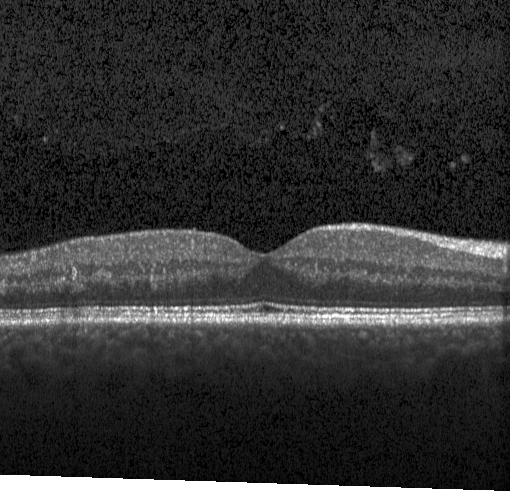 Heidelberg Spectralis OCT system; OCT line scan; spectral-domain optical coherence tomography; centered on the fovea. The scan shows no choroidal neovascularization, diabetic macular edema, or drusen.